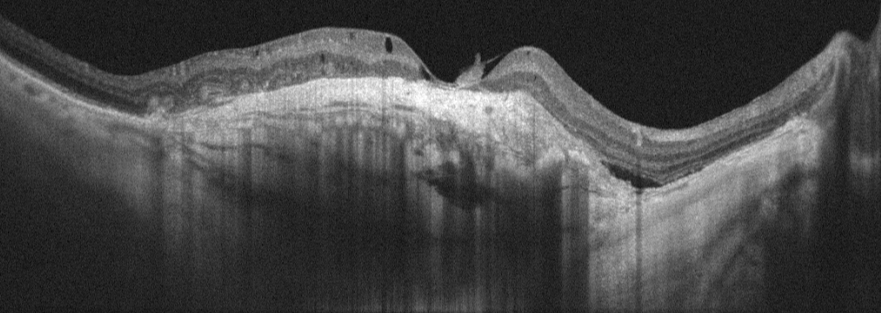 Retinal OCT cross-section. Through the macula. Dx: age-related macular degeneration (AMD).